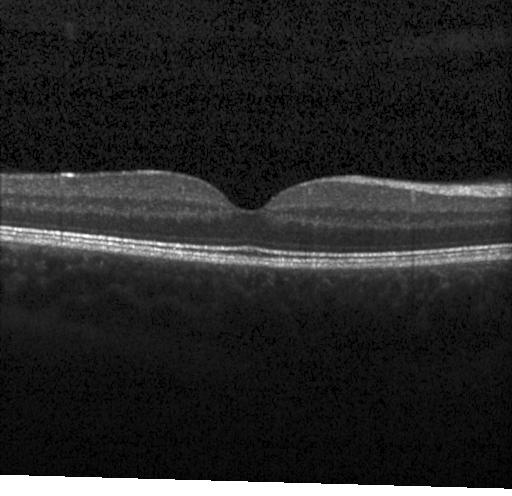

Finding: neither choroidal neovascularization, diabetic macular edema, nor drusen.